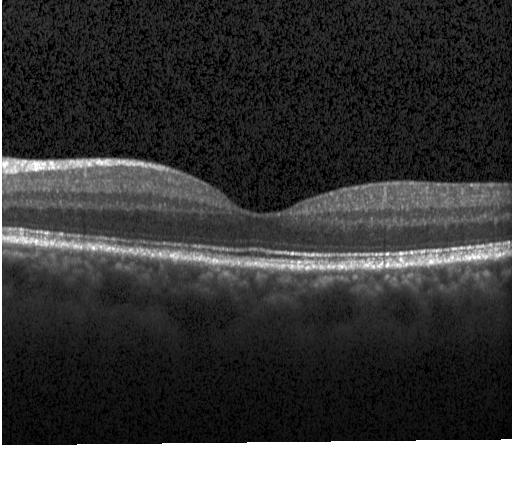

OCT line scan; spectral-domain OCT — This B-scan demonstrates no CNV, DME, or drusen.